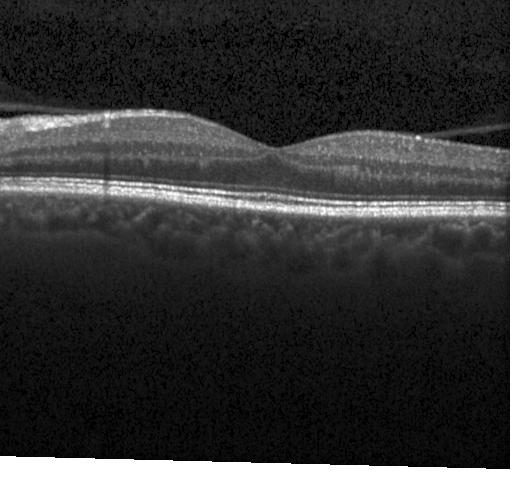 Retinal OCT cross-section. Spectral-domain optical coherence tomography. Macular scan
Macular OCT: neither choroidal neovascularization, diabetic macular edema, nor drusen.